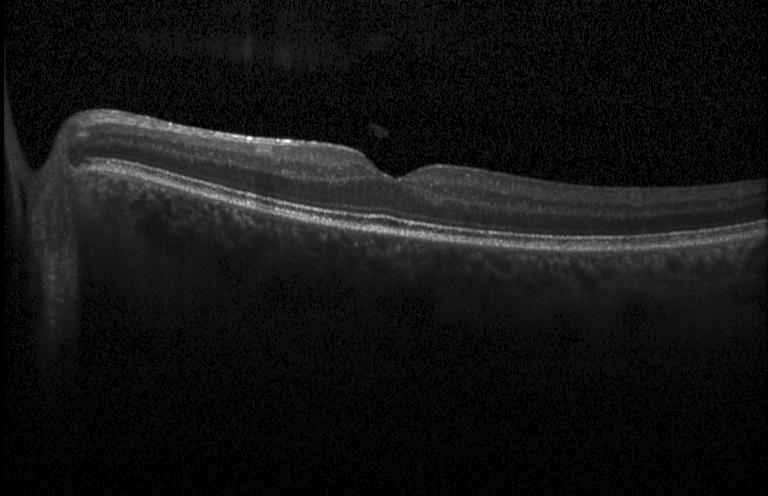

Optical coherence tomography B-scan. Macular scan
Macular OCT: no evidence of CNV, DME, or drusen.